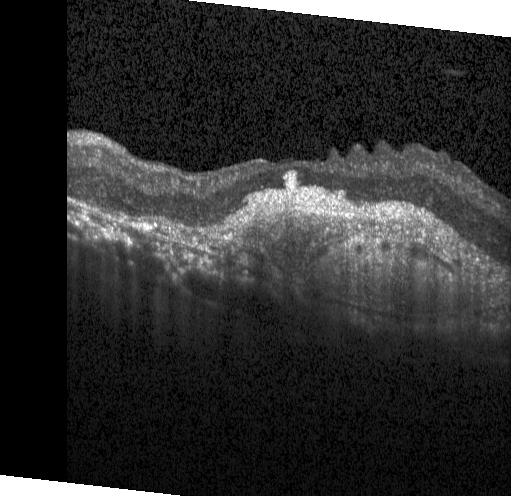
Retinal OCT cross-section; spectral-domain OCT.
Diagnosis: choroidal neovascularization.